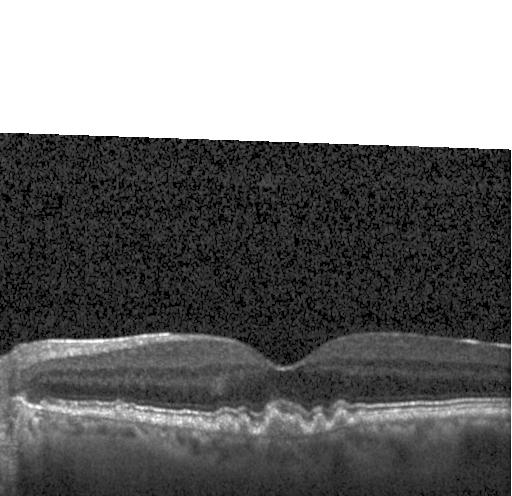
Spectral-domain OCT B-scan: sub-RPE drusenoid deposits.